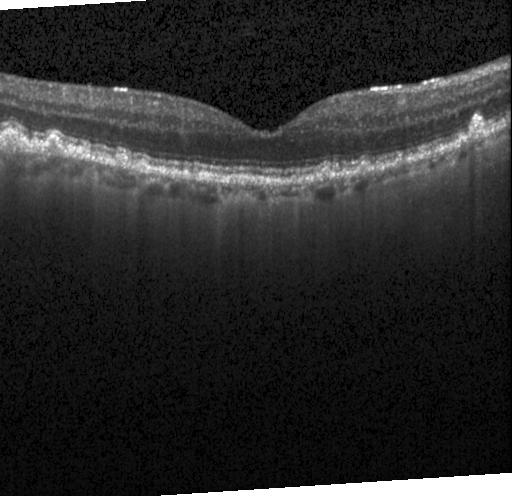

Impression: sub-RPE drusenoid deposits.